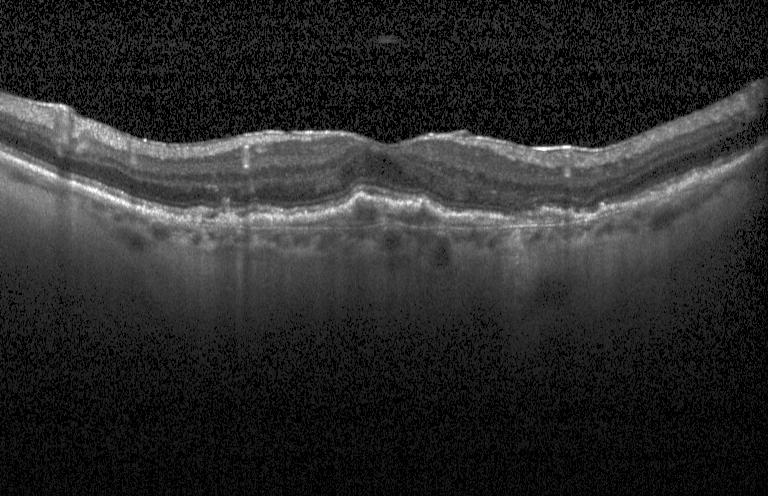

Impression: CNV.